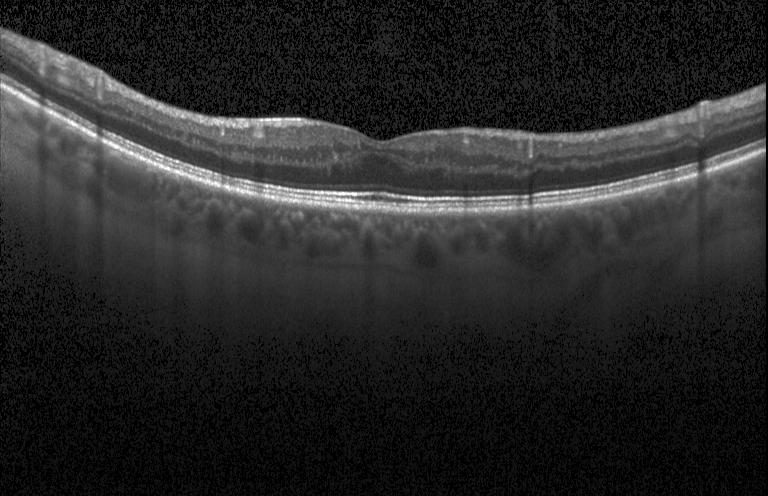 OCT B-scan.
Assessment: no evidence of CNV, DME, or drusen.